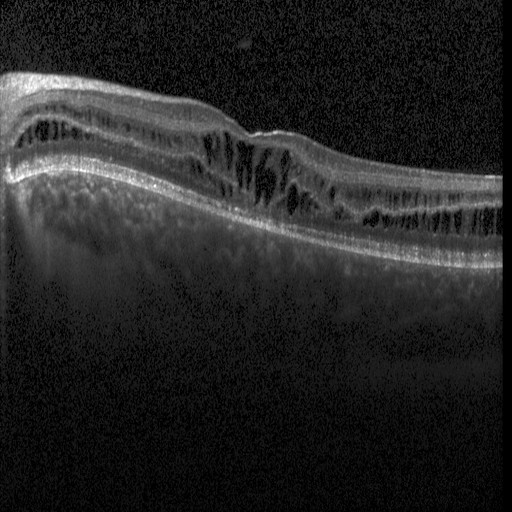 This B-scan demonstrates diabetic macular edema.